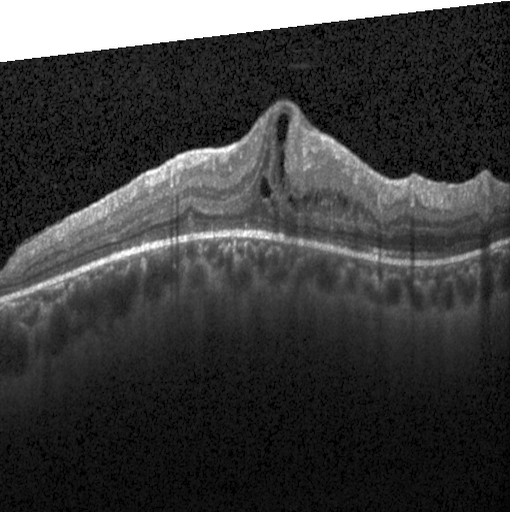
Heidelberg Spectralis OCT system, retinal OCT cross-section, SD-OCT, horizontal scan through the fovea. Diagnosis: diabetic macular edema (DME).